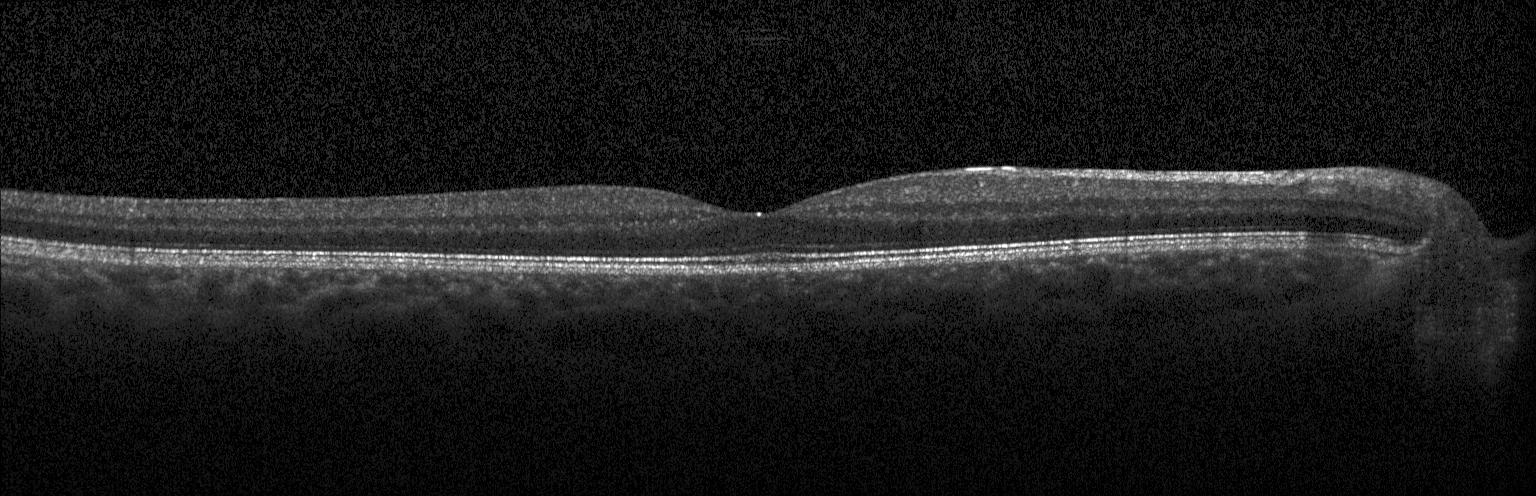 OCT scan showing neither choroidal neovascularization, diabetic macular edema, nor drusen.